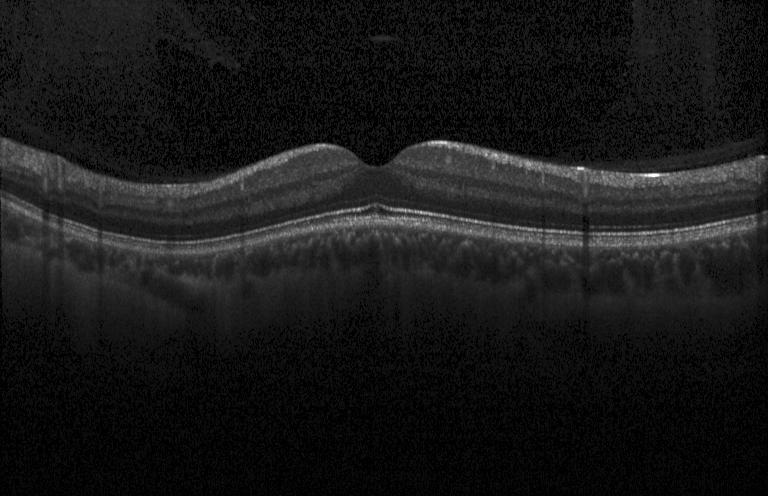
Heidelberg Spectralis OCT system, optical coherence tomography scan, horizontal scan through the fovea. Diagnosis: no evidence of choroidal neovascularization, diabetic macular edema, or drusen.